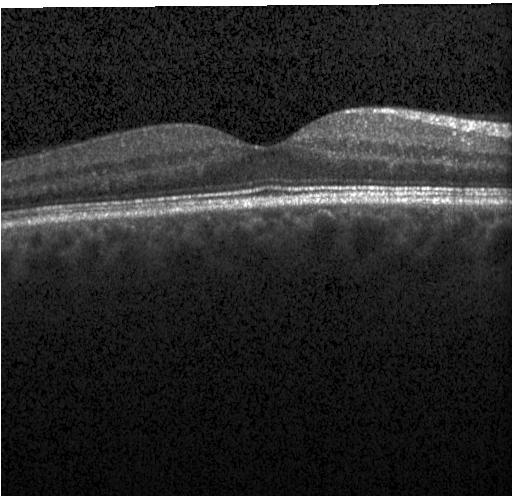

Optical coherence tomography B-scan, SD-OCT, Heidelberg Spectralis OCT system, macular scan.
Diagnosis: neither choroidal neovascularization, diabetic macular edema, nor drusen.